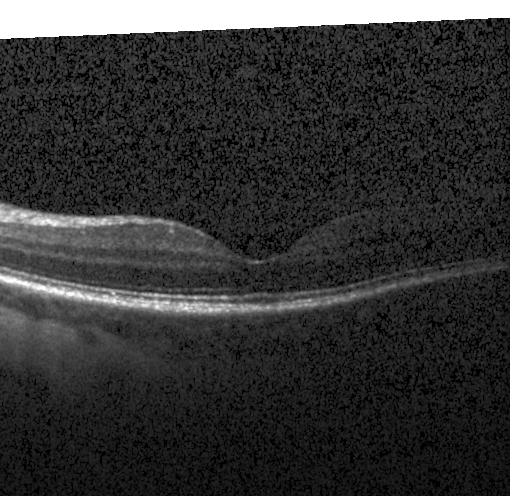
Fovea-centered · SD-OCT · optical coherence tomography scan · Heidelberg Spectralis OCT system
Assessment: no choroidal neovascularization, diabetic macular edema, or drusen.